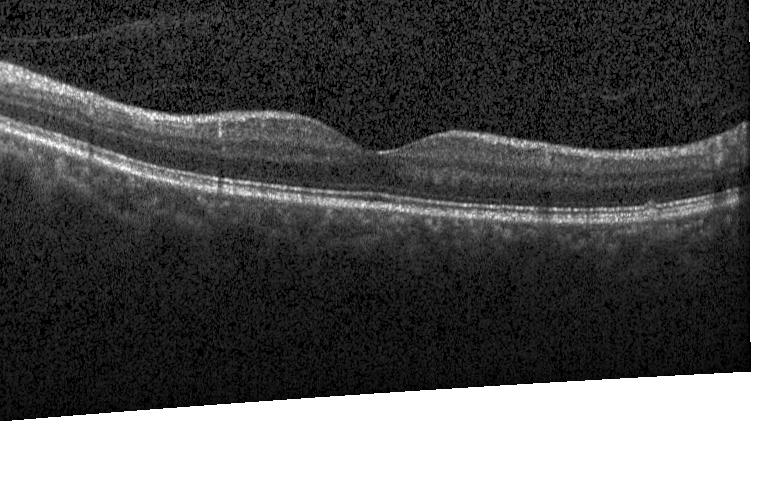 Impression: neither choroidal neovascularization, diabetic macular edema, nor drusen.